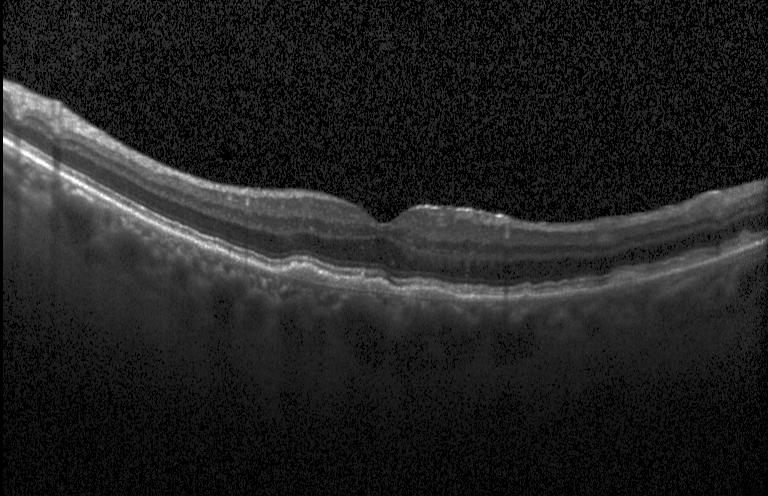

Spectral-domain optical coherence tomography, macular scan, OCT B-scan, Heidelberg Spectralis. A choroidal neovascular membrane.